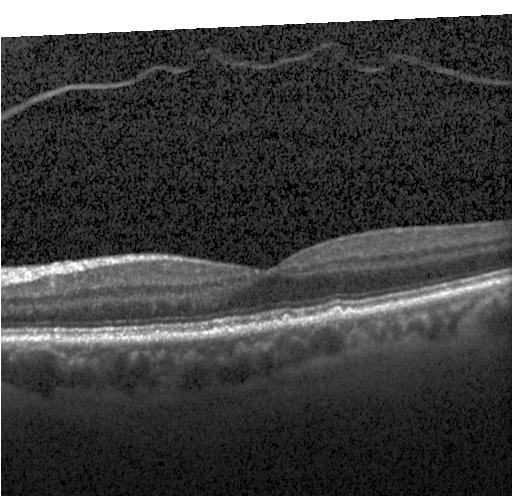 Dx: sub-RPE drusenoid deposits.